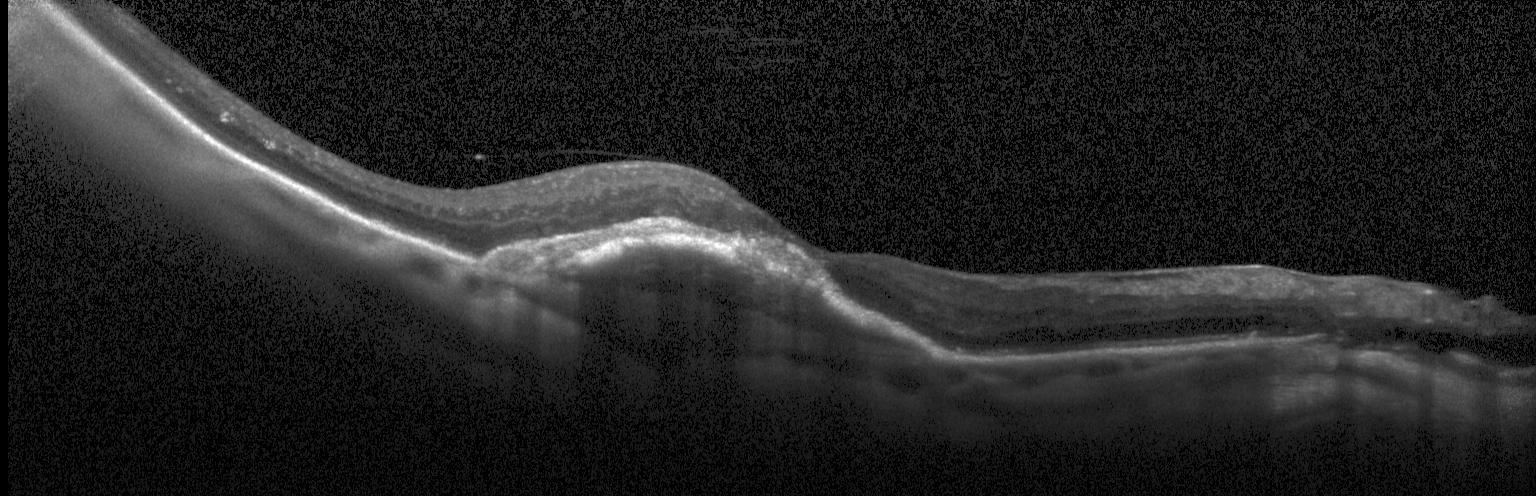
Assessment: a choroidal neovascular membrane.